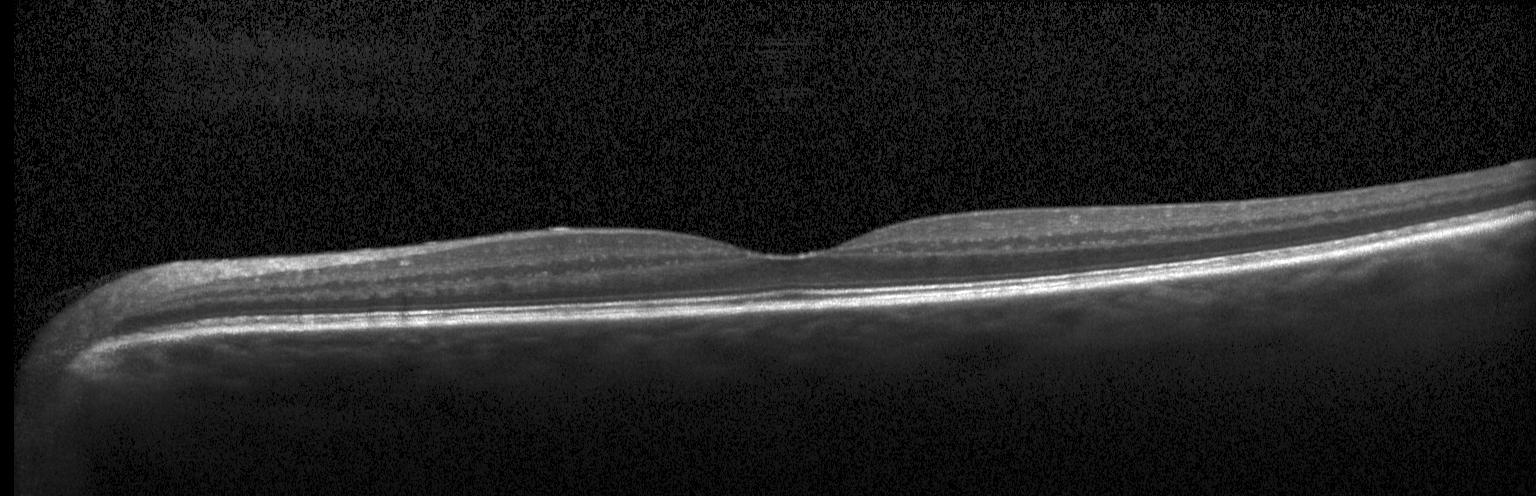

Retinal OCT cross-section · centered on the fovea · SD-OCT · acquired on a Heidelberg Spectralis.
Finding: no choroidal neovascularization, diabetic macular edema, or drusen.